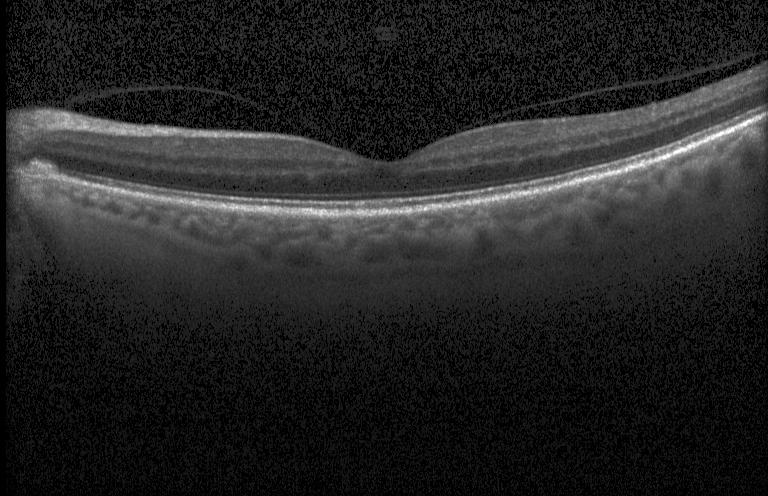 Impression: no CNV, no DME, and no drusen.